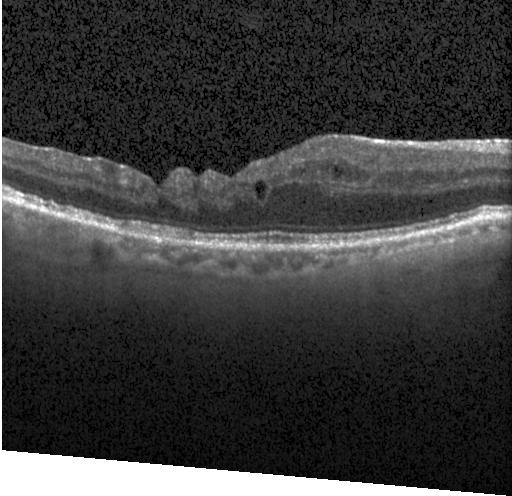

Spectral-domain OCT B-scan: diabetic macular edema (DME).